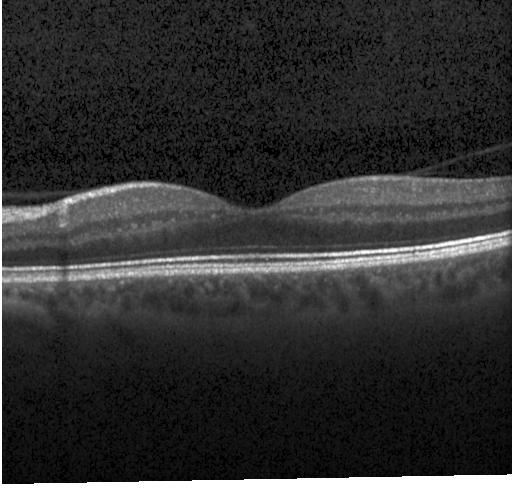

Optical coherence tomography B-scan, SD-OCT, horizontal scan through the fovea
Finding: no evidence of choroidal neovascularization, diabetic macular edema, or drusen.